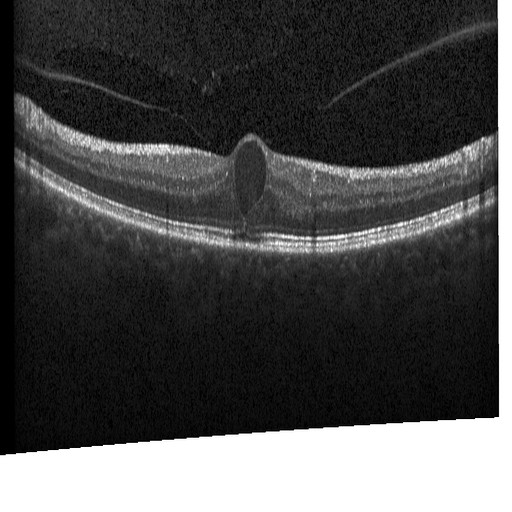

OCT B-scan.
Assessment: diabetic macular edema.